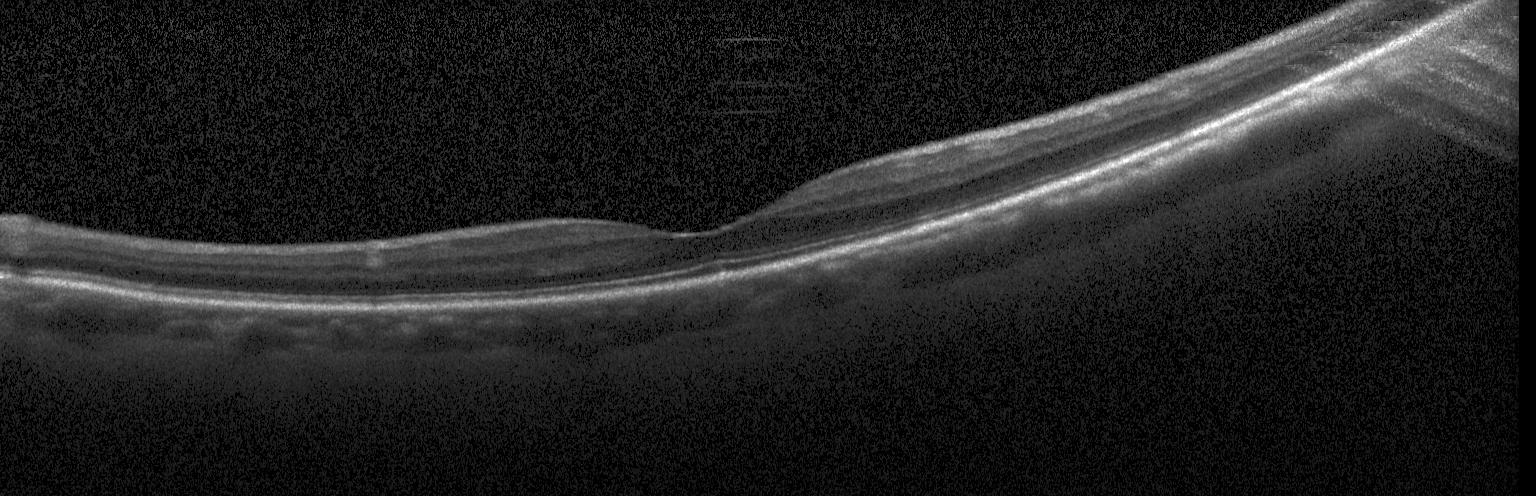
Centered on the fovea. Spectral-domain optical coherence tomography. Acquired on a Heidelberg Spectralis. Optical coherence tomography B-scan — Impression: no CNV, DME, or drusen.